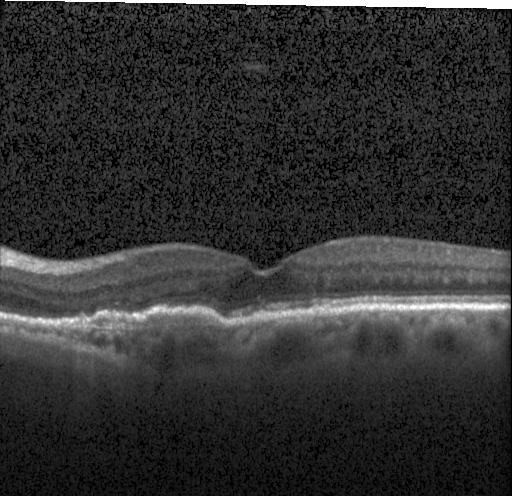 Spectral-domain optical coherence tomography. Acquired on a Heidelberg Spectralis. OCT B-scan — A choroidal neovascular membrane.